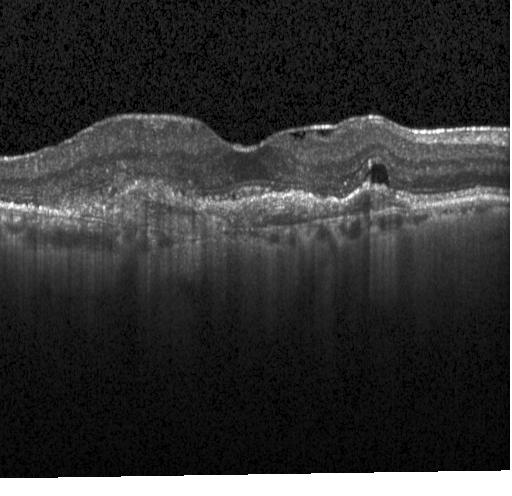 Optical coherence tomography scan.
This B-scan demonstrates choroidal neovascularization (CNV).